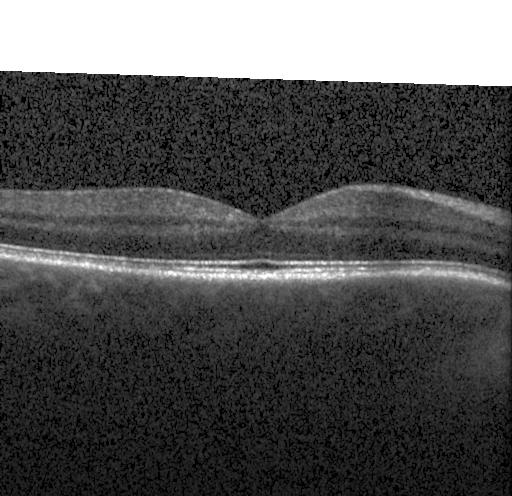 Retinal OCT B-scan. Spectral-domain optical coherence tomography. Heidelberg Spectralis
No CNV, DME, or drusen.